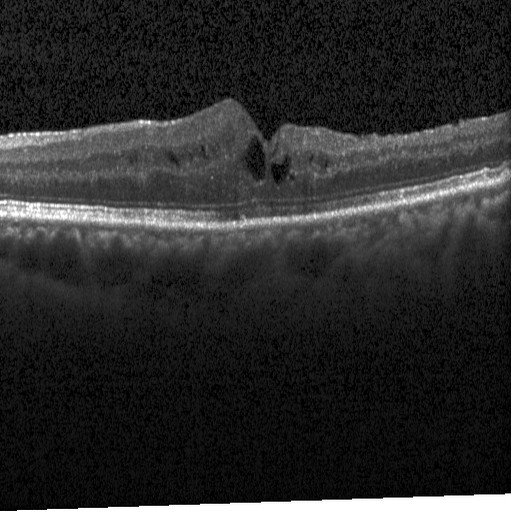 Assessment: DME.